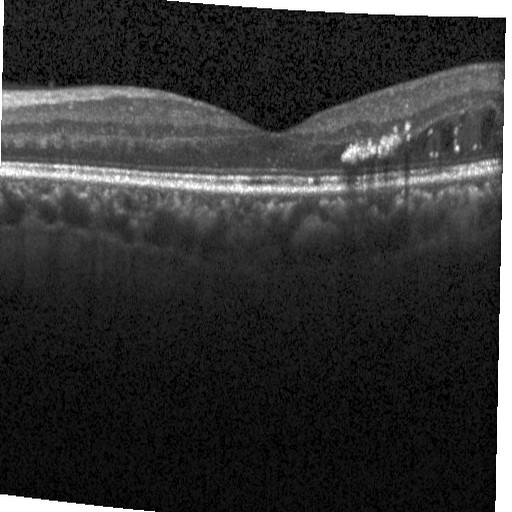 Optical coherence tomography B-scan, instrument: Heidelberg Spectralis
Finding: diabetic macular edema.